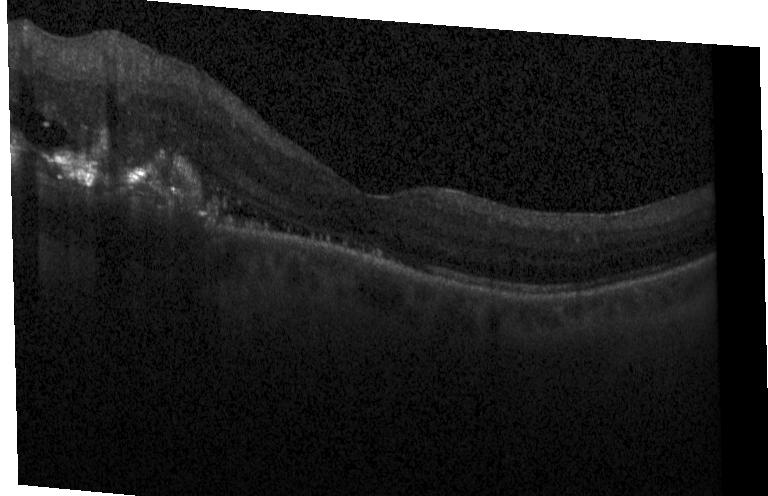
Retinal OCT cross-section. The scan shows choroidal neovascularization.